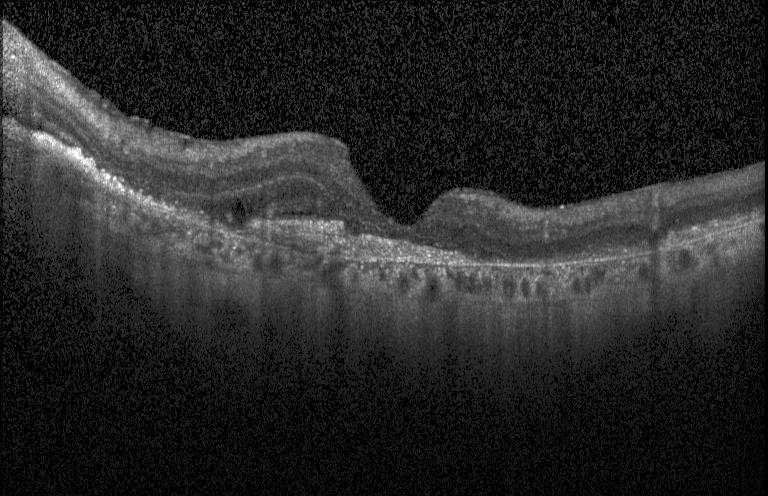

OCT B-scan. OCT finding: CNV.